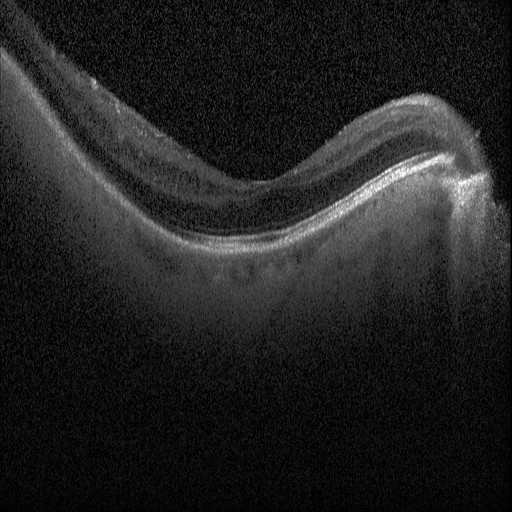 Diabetic macular edema (DME).